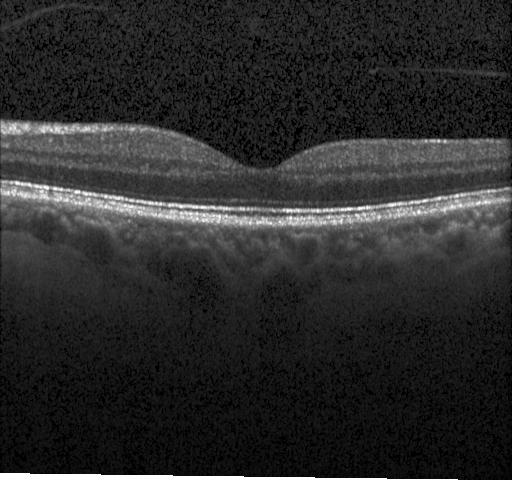
Spectral-domain OCT, OCT B-scan, Heidelberg Spectralis OCT system, horizontal scan through the fovea.
Diagnosis: no choroidal neovascularization, no diabetic macular edema, and no drusen.